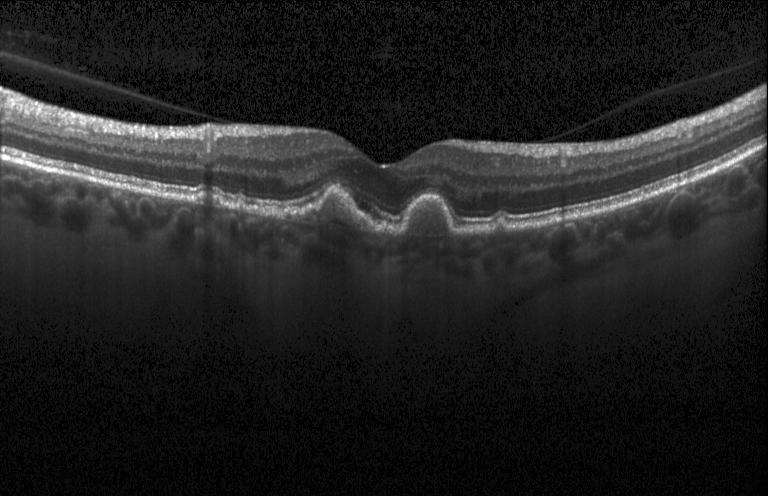

OCT line scan.
Diagnosis: sub-RPE drusenoid deposits.